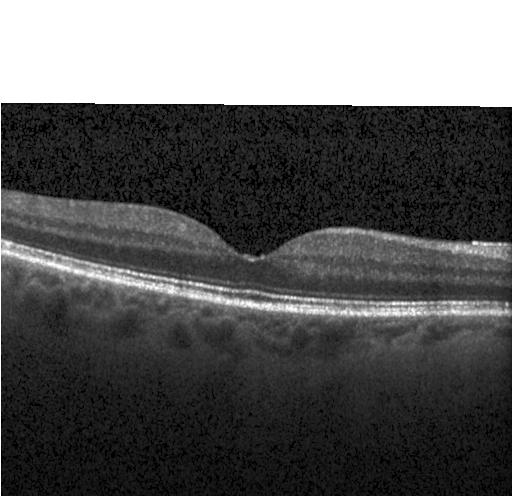
Spectral-domain OCT · optical coherence tomography B-scan · through the macula
Finding: no evidence of CNV, DME, or drusen.